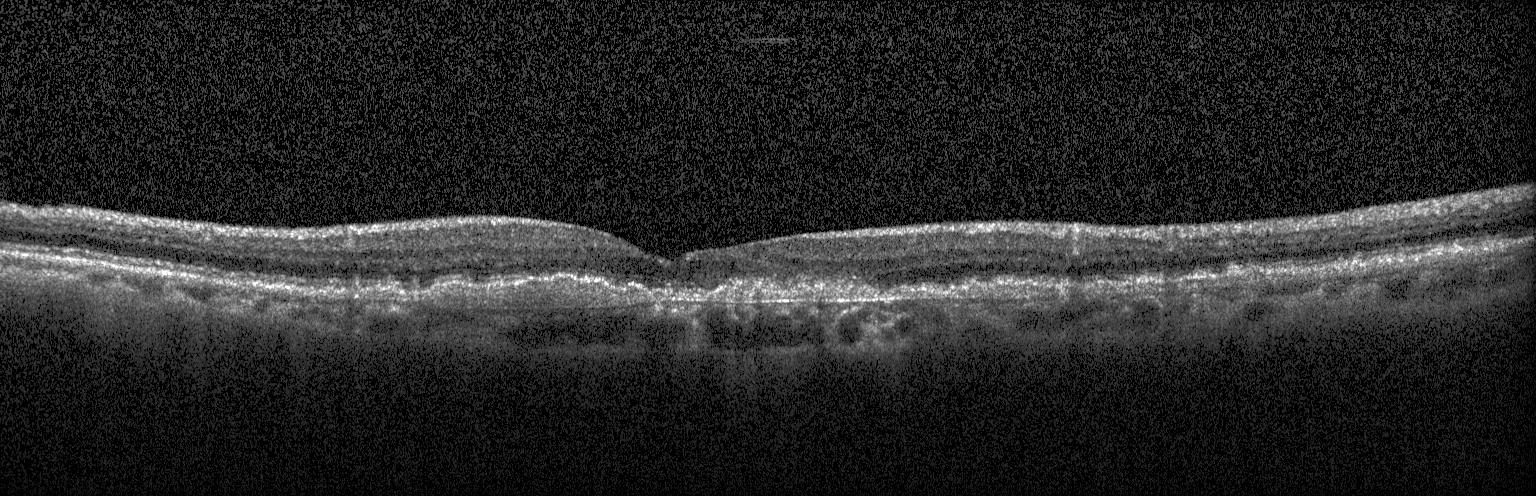
Optical coherence tomography scan · Heidelberg Spectralis OCT system — The scan shows a choroidal neovascular membrane.